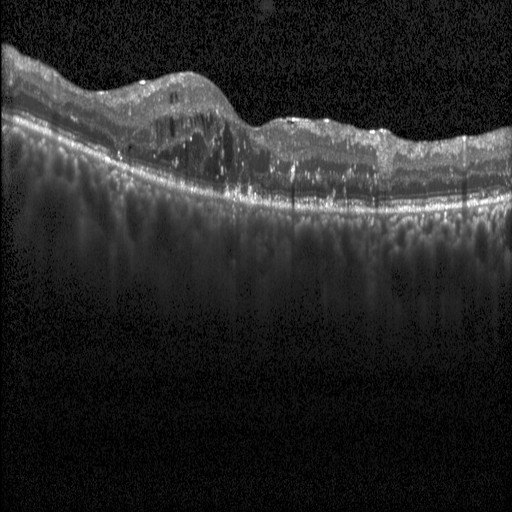 Acquired on a Heidelberg Spectralis, spectral-domain optical coherence tomography, OCT B-scan, fovea-centered. Impression: DME.